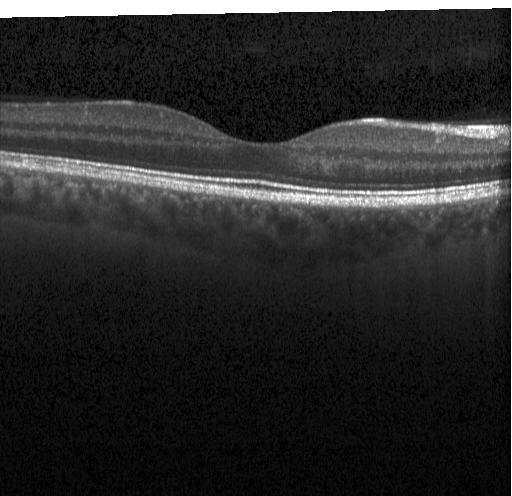 Retinal OCT cross-section; Heidelberg Spectralis OCT system; through the macula — Diagnosis: no evidence of choroidal neovascularization, diabetic macular edema, or drusen.